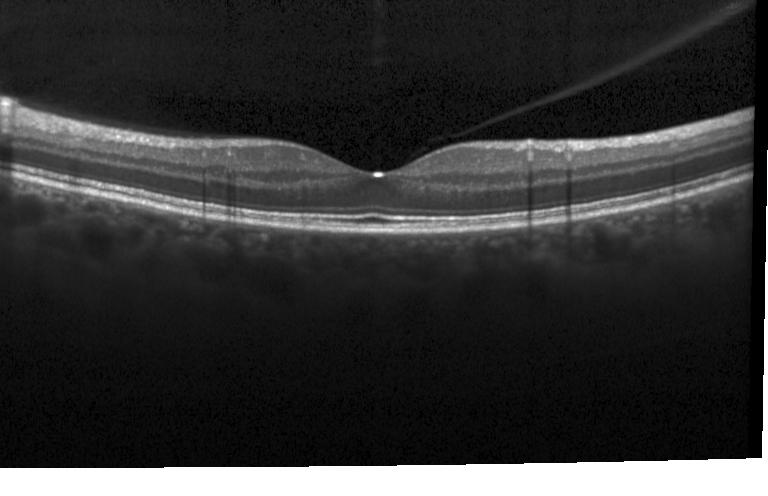
Impression: no evidence of choroidal neovascularization, diabetic macular edema, or drusen.